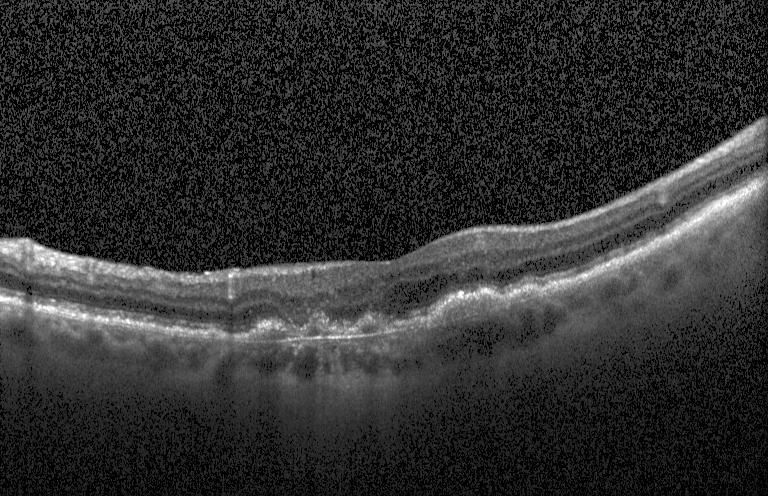

Dx: a choroidal neovascular membrane.